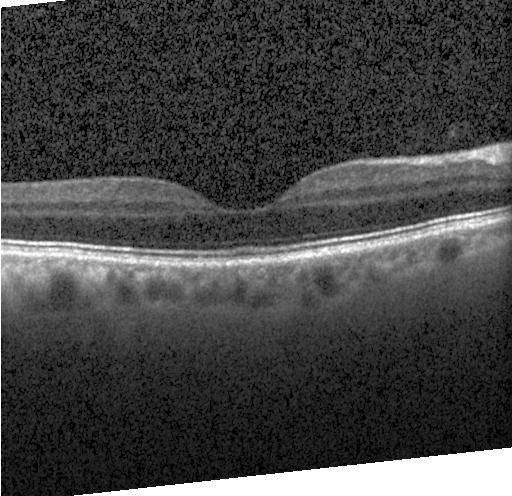
Impression: no choroidal neovascularization, diabetic macular edema, or drusen.